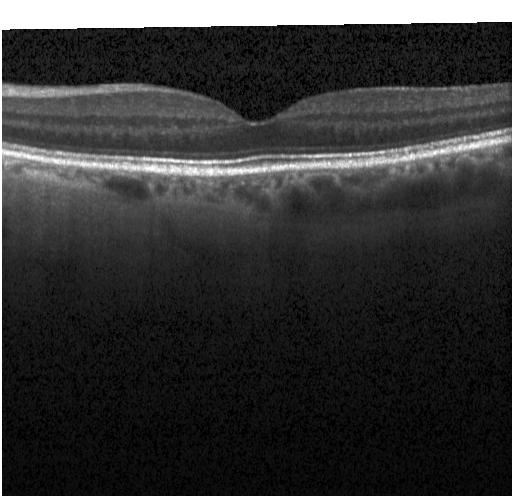

SD-OCT; optical coherence tomography B-scan
Impression: neither choroidal neovascularization, diabetic macular edema, nor drusen.